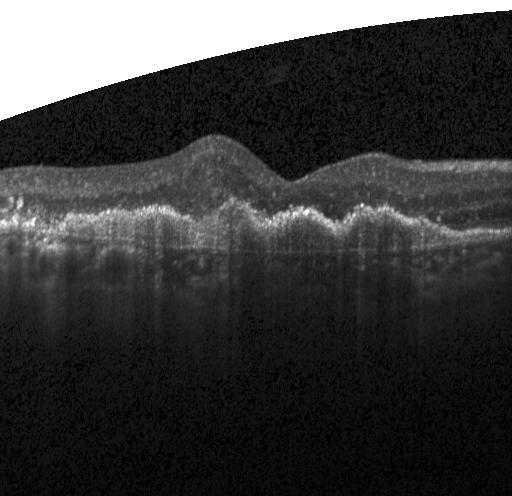
Retinal OCT B-scan; instrument: Heidelberg Spectralis — This B-scan demonstrates a choroidal neovascular membrane.